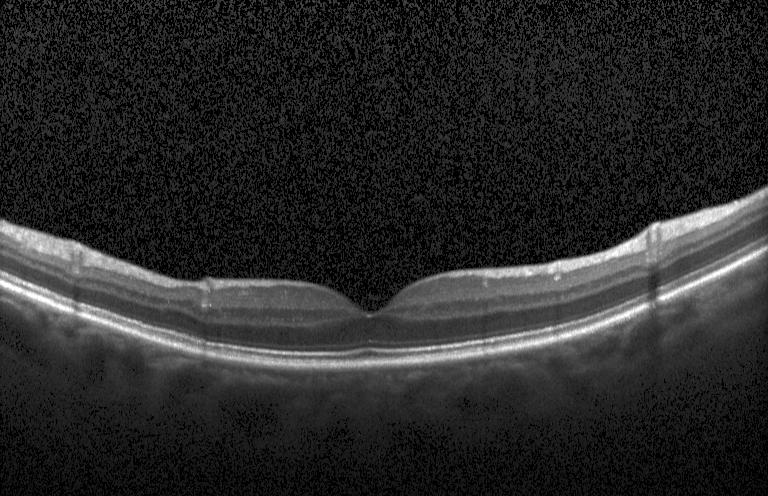

Macular OCT: neither CNV, DME, nor drusen.